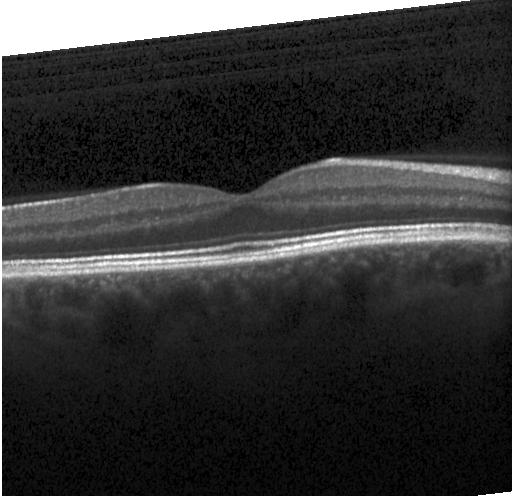
OCT B-scan
This B-scan demonstrates no CNV, DME, or drusen.